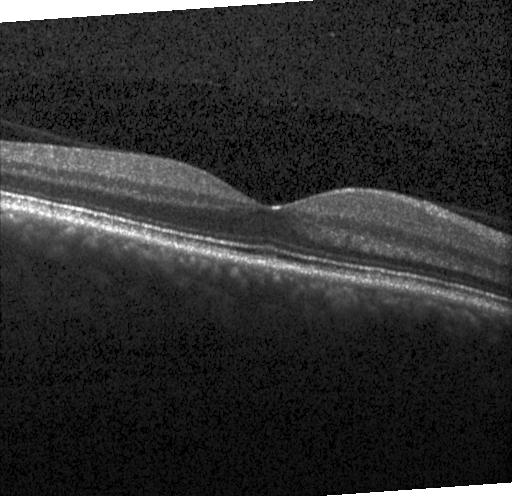
OCT B-scan showing no choroidal neovascularization, no diabetic macular edema, and no drusen.